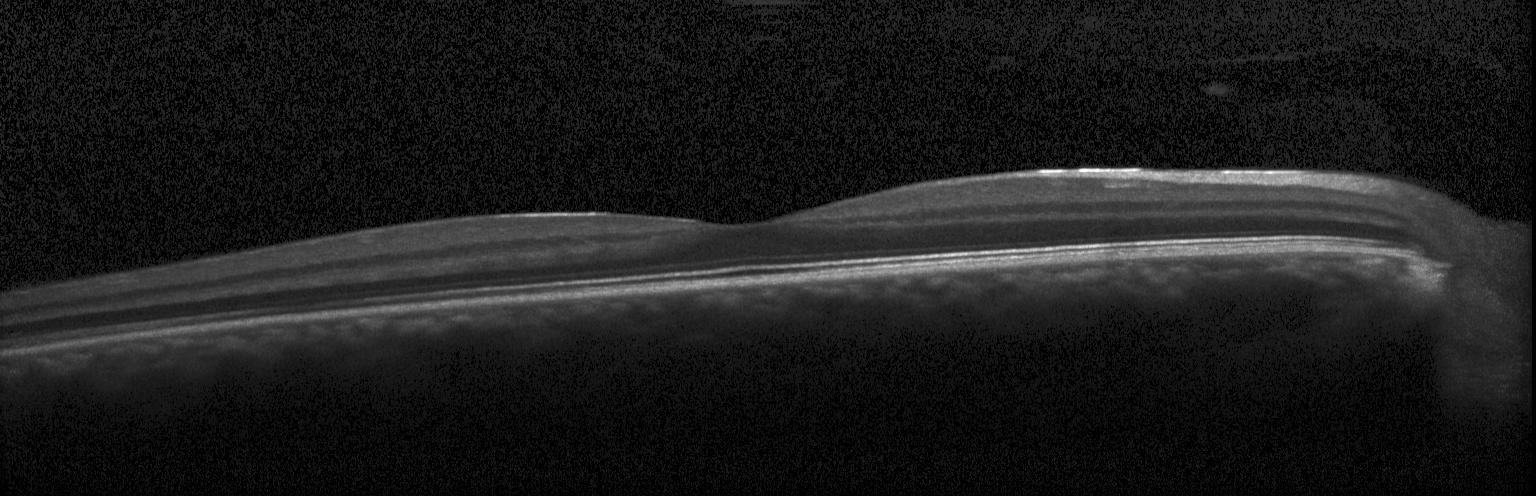

Spectral-domain OCT B-scan: no evidence of choroidal neovascularization, diabetic macular edema, or drusen.